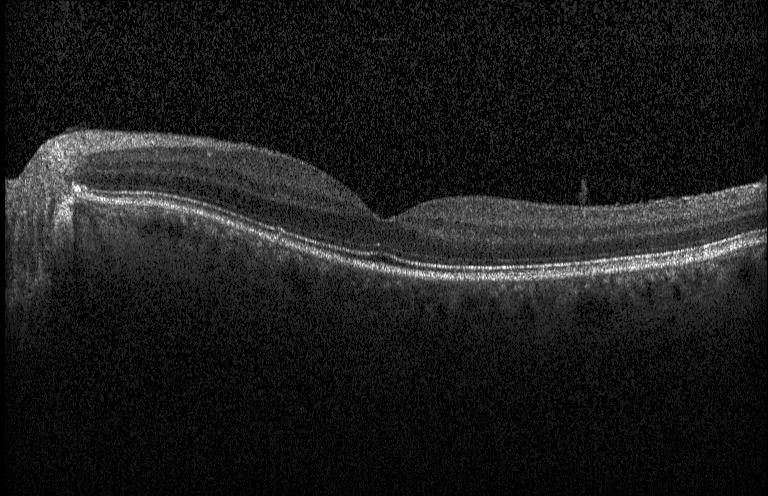

Macular OCT demonstrating neither choroidal neovascularization, diabetic macular edema, nor drusen.